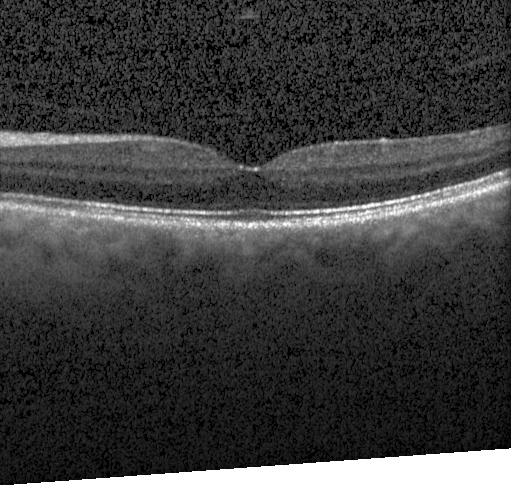 Dx: no evidence of CNV, DME, or drusen.